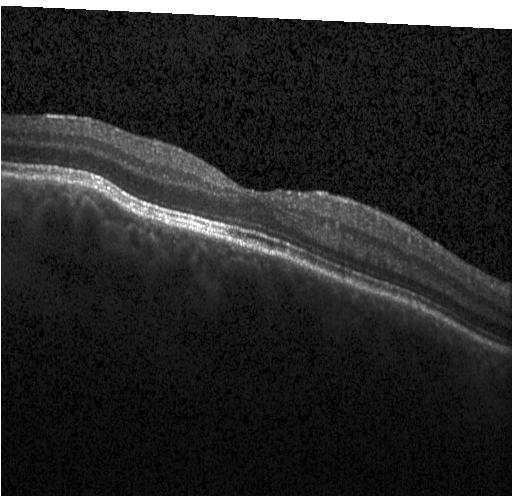 Instrument: Heidelberg Spectralis. Spectral-domain OCT. Retinal OCT cross-section. Centered on the fovea. OCT finding: neither CNV, DME, nor drusen.